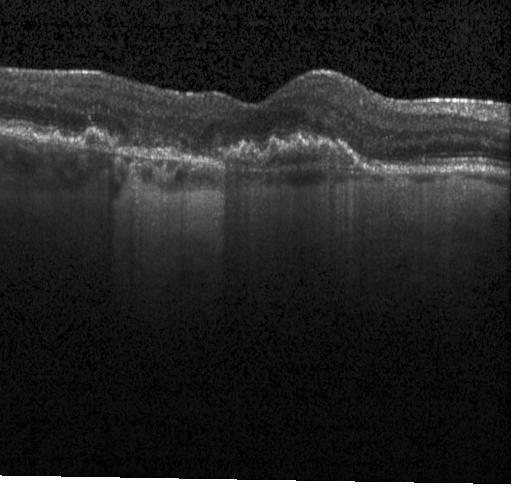
Fovea-centered · optical coherence tomography B-scan · SD-OCT — This B-scan demonstrates a choroidal neovascular membrane.